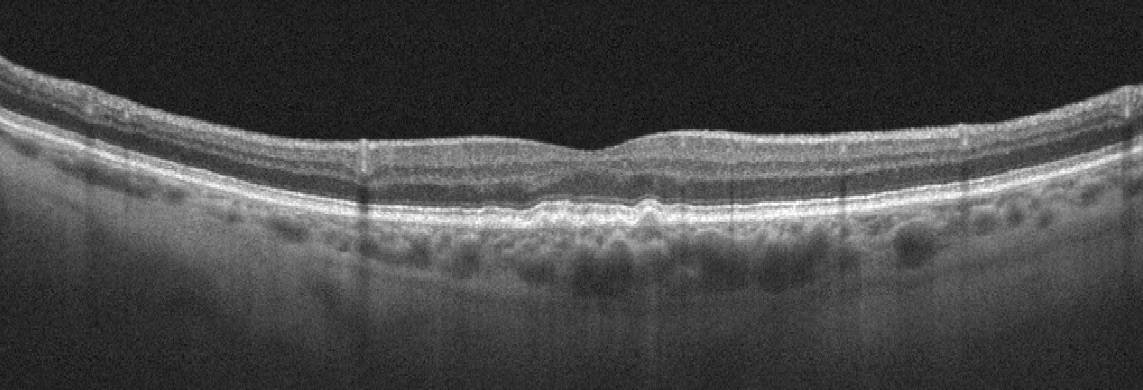

OCT line scan. Assessment: age-related macular degeneration.